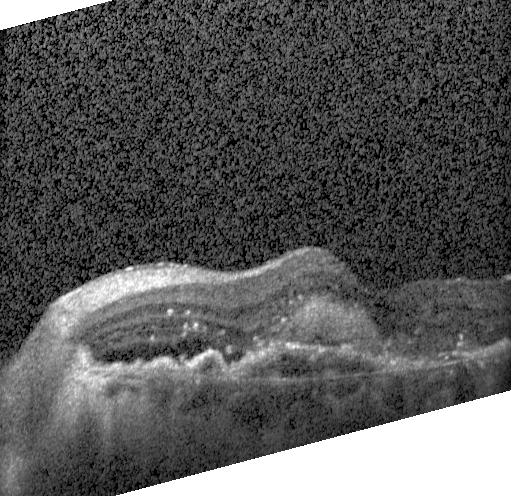 OCT B-scan. OCT finding: a choroidal neovascular membrane.